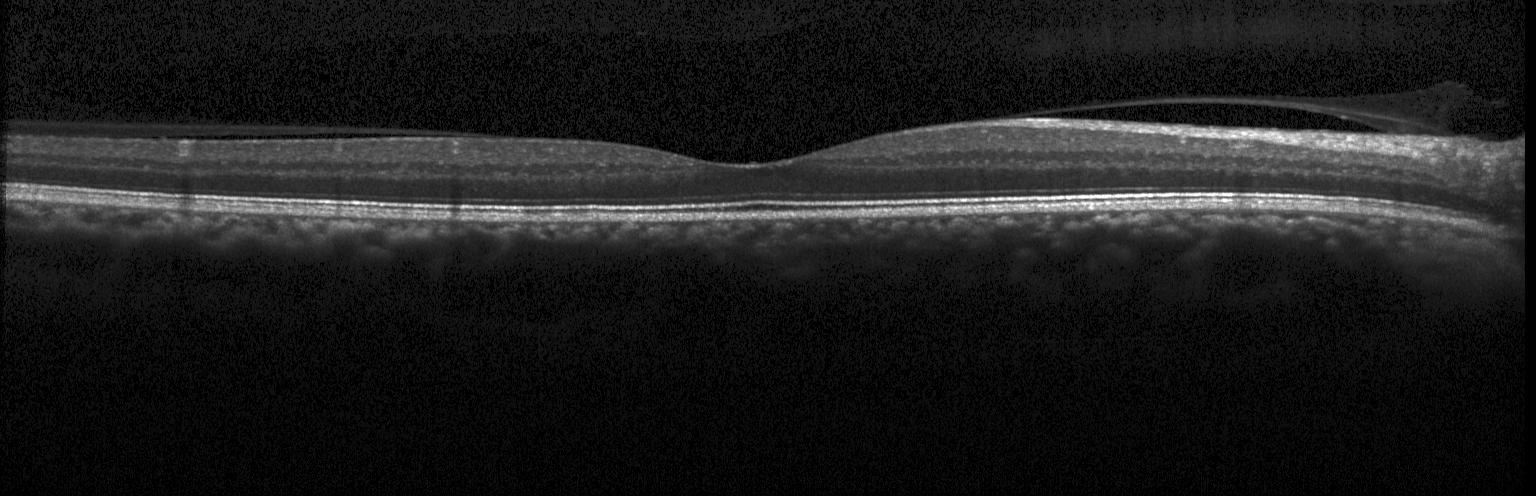
Impression: neither choroidal neovascularization, diabetic macular edema, nor drusen.